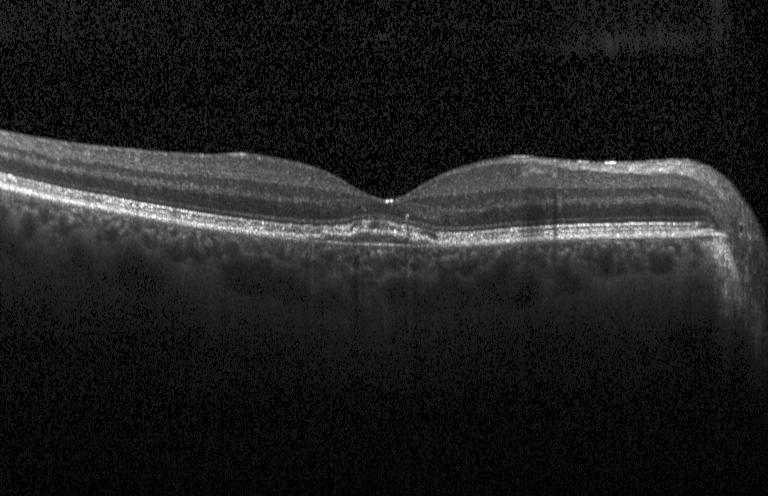

Retinal OCT B-scan, centered on the fovea.
Macular OCT: a choroidal neovascular membrane.